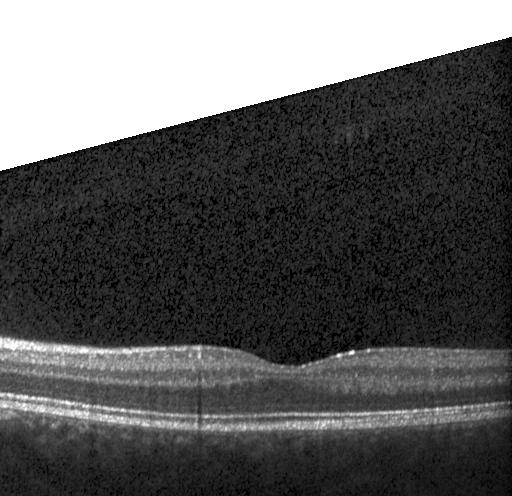 Diagnosis: no CNV, no DME, and no drusen.